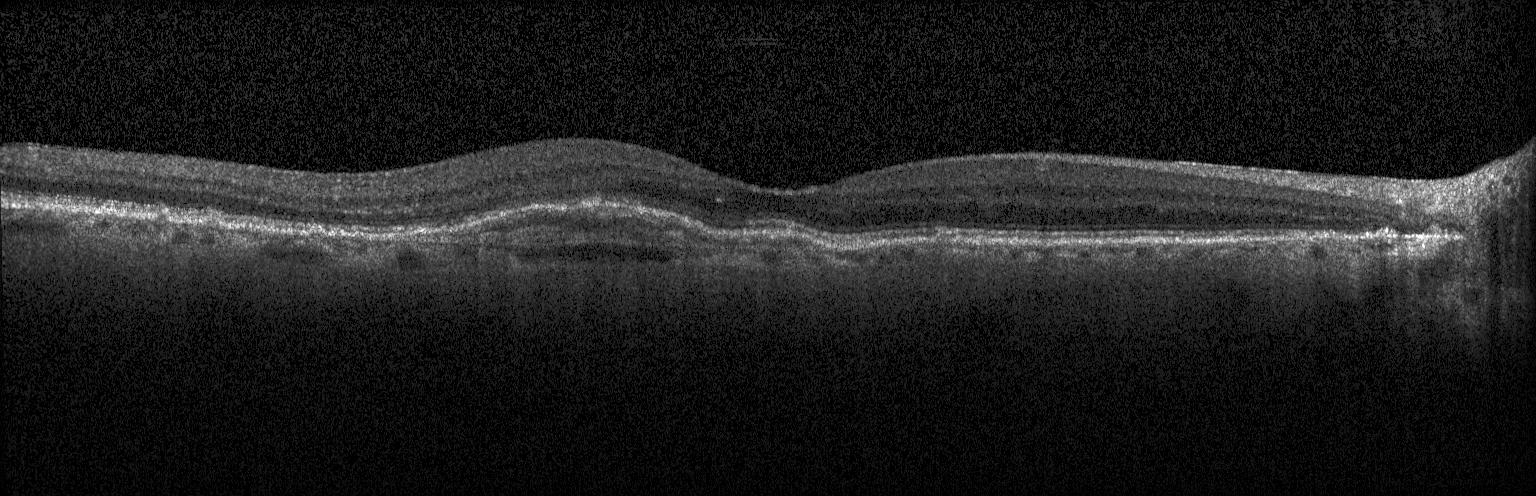 OCT B-scan, spectral-domain OCT, centered on the fovea.
The scan shows CNV.